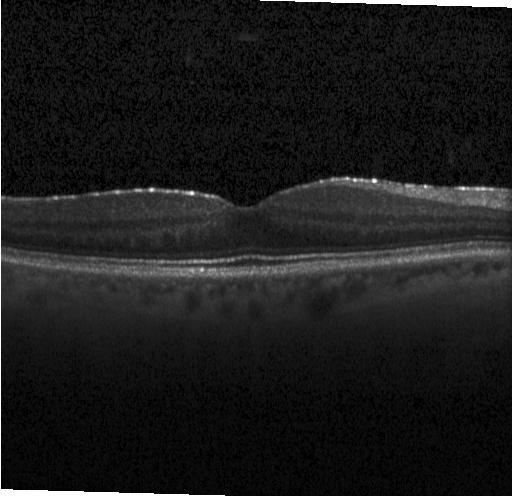 Spectral-domain OCT, OCT B-scan. Diagnosis: no choroidal neovascularization, no diabetic macular edema, and no drusen.